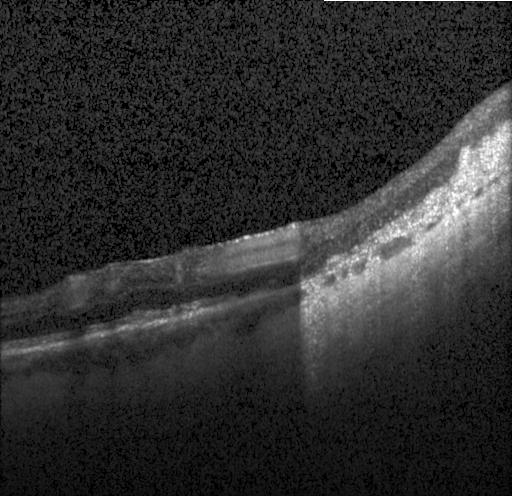
Impression: a choroidal neovascular membrane.